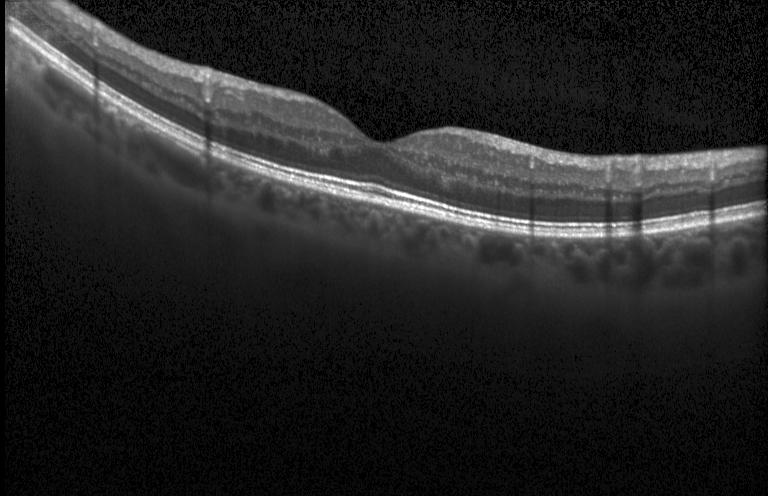

OCT line scan, centered on the fovea, instrument: Heidelberg Spectralis — Finding: neither CNV, DME, nor drusen.